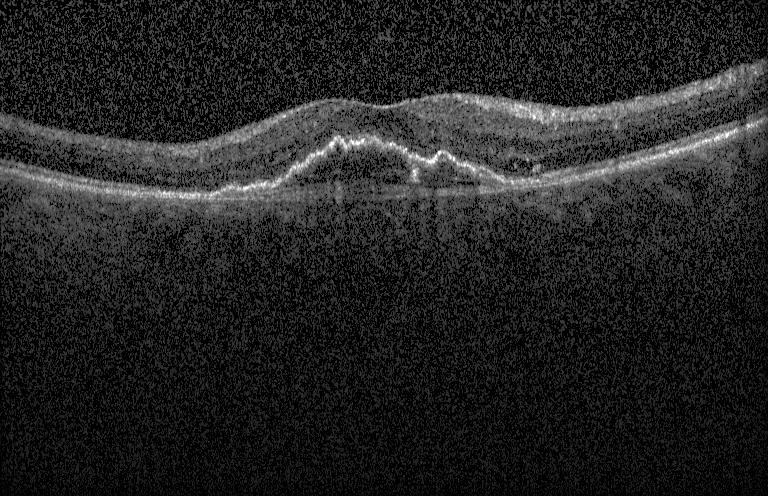 Retinal OCT cross-section. Acquired on a Heidelberg Spectralis — Diagnosis: a choroidal neovascular membrane.